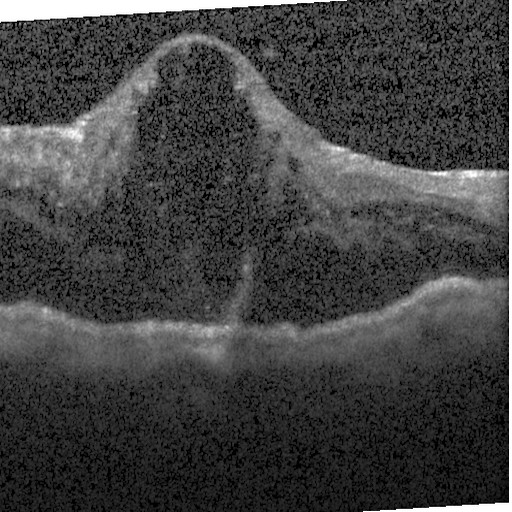 OCT B-scan, spectral-domain optical coherence tomography, fovea-centered, instrument: Heidelberg Spectralis.
Diagnosis: DME.